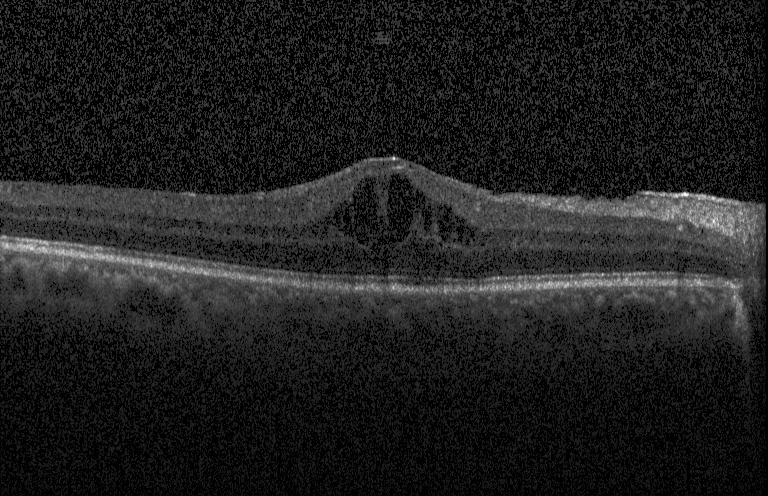
OCT B-scan showing diabetic macular edema (DME).